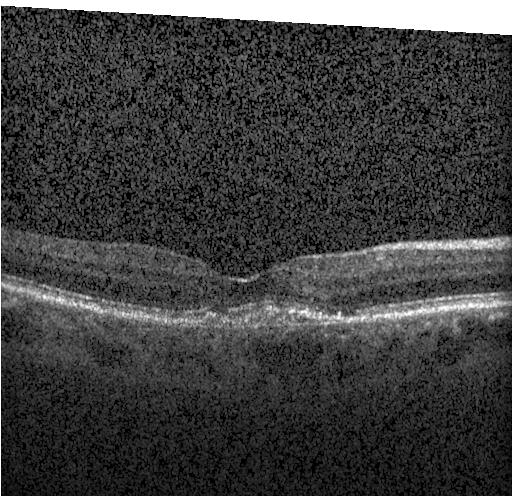
Spectral-domain optical coherence tomography, fovea-centered, retinal OCT cross-section, acquired on a Heidelberg Spectralis — Diagnosis: choroidal neovascularization (CNV).